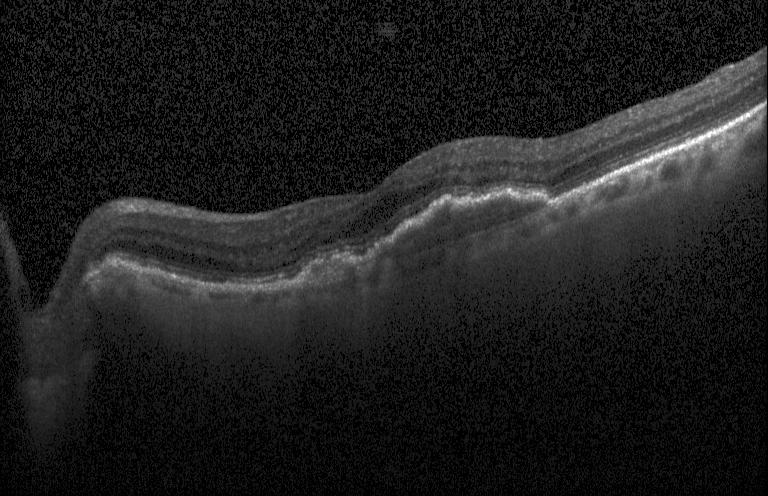
Dx: CNV.